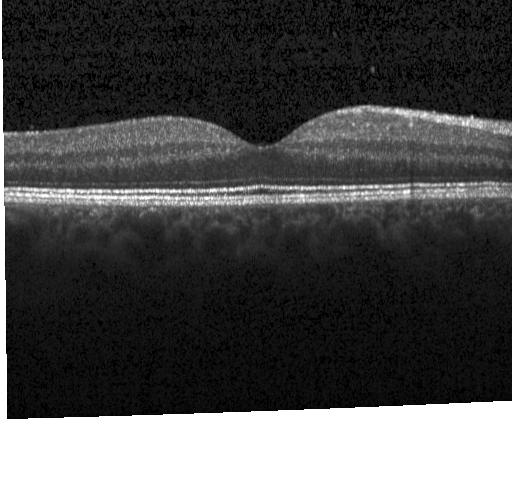 Optical coherence tomography B-scan · centered on the fovea · Heidelberg Spectralis — The scan shows no CNV, DME, or drusen.